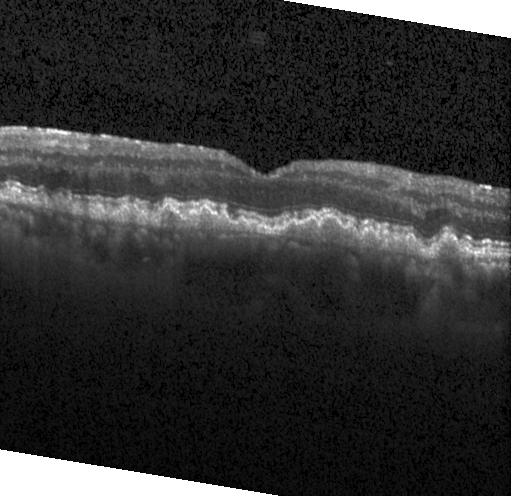
Retinal OCT B-scan
OCT finding: CNV.